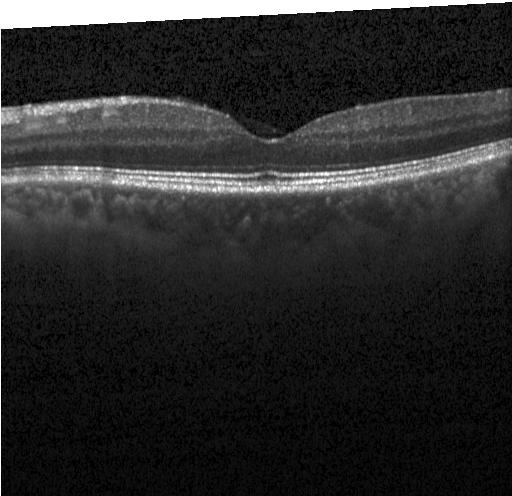 OCT B-scan
OCT finding: no choroidal neovascularization, diabetic macular edema, or drusen.